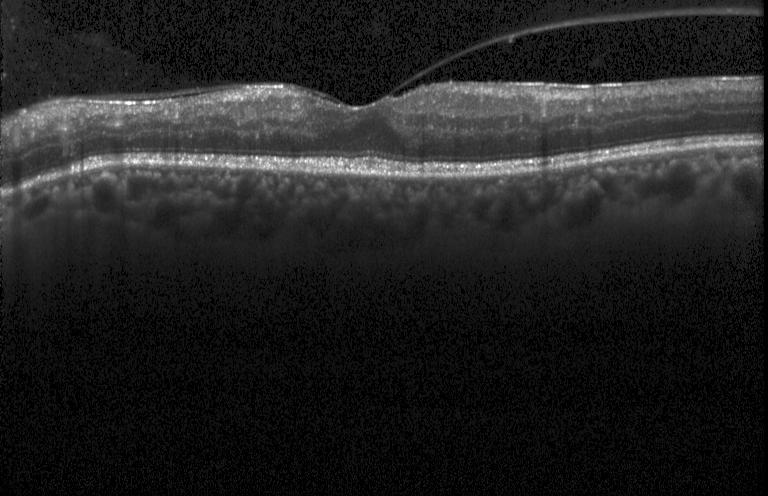

Dx: diabetic macular edema (DME).